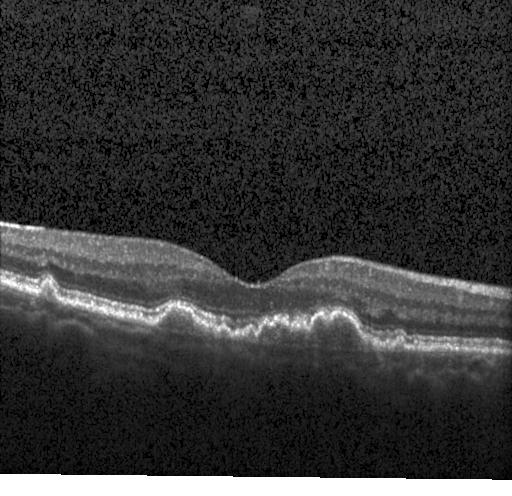

Optical coherence tomography scan. Heidelberg Spectralis OCT system. Centered on the fovea. SD-OCT
Dx: multiple drusen.